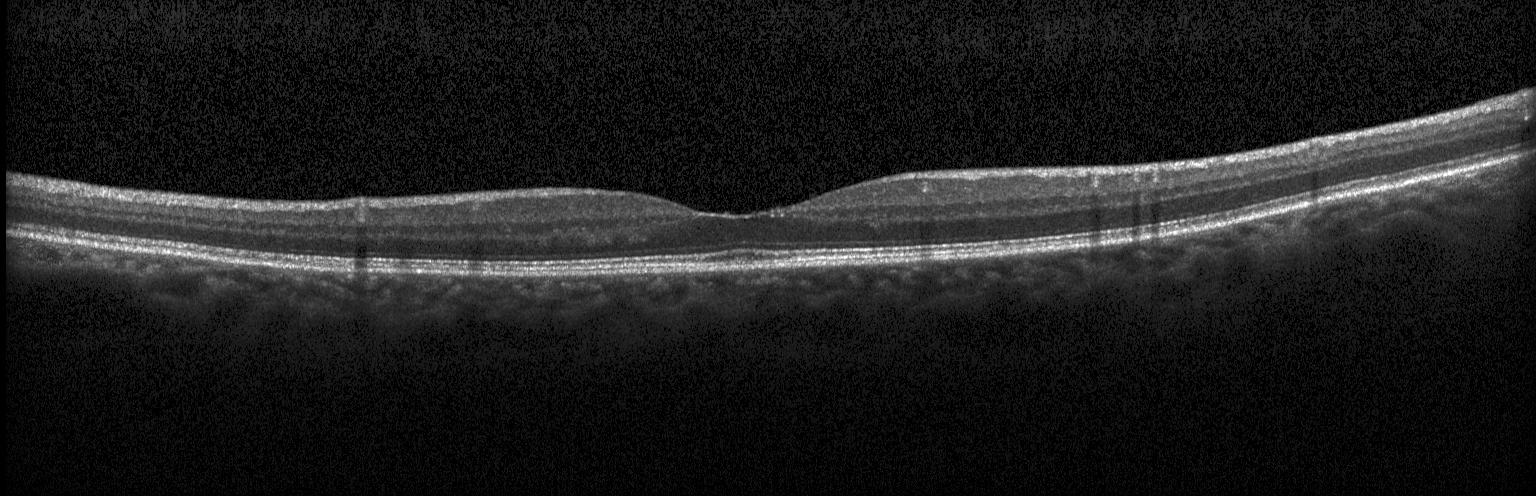
Retinal OCT B-scan.
Finding: neither choroidal neovascularization, diabetic macular edema, nor drusen.